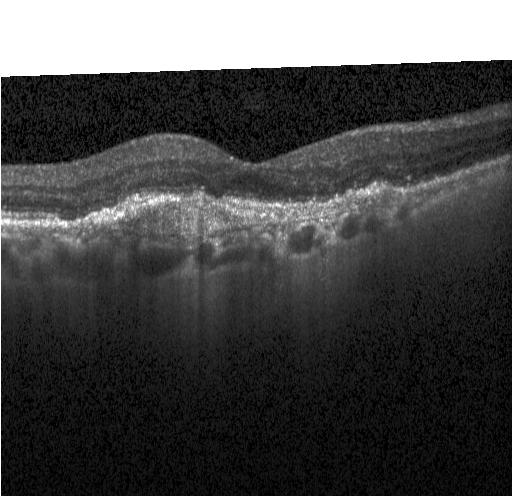 OCT B-scan; SD-OCT
Impression: a choroidal neovascular membrane.